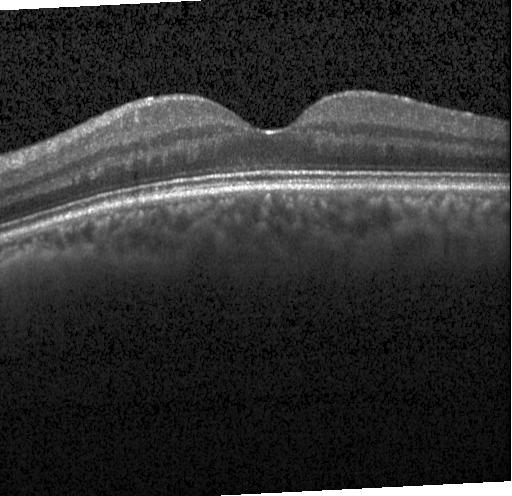 Spectral-domain OCT; retinal OCT cross-section; through the macula
Impression: no choroidal neovascularization, diabetic macular edema, or drusen.